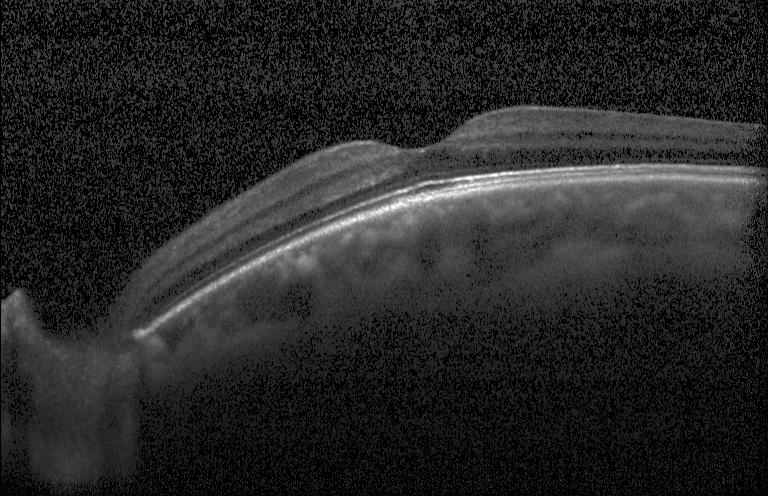

Optical coherence tomography scan. Finding: neither choroidal neovascularization, diabetic macular edema, nor drusen.